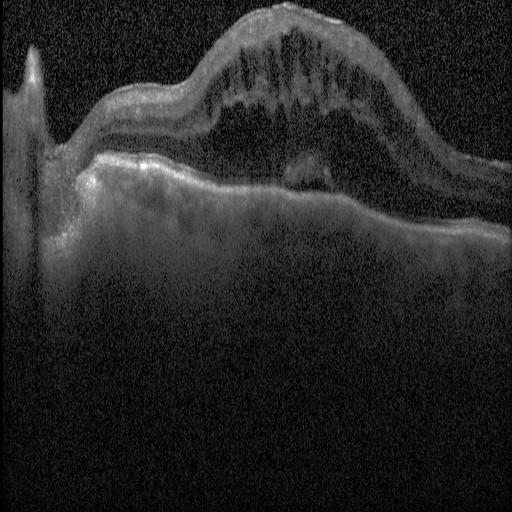
Horizontal scan through the fovea. Spectral-domain optical coherence tomography. Heidelberg Spectralis. Optical coherence tomography B-scan
Finding: DME.